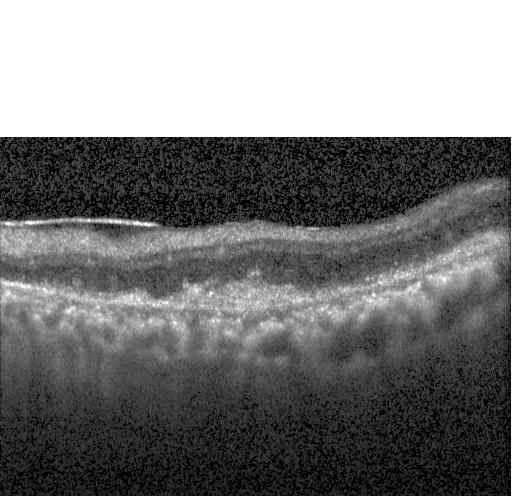 A choroidal neovascular membrane.